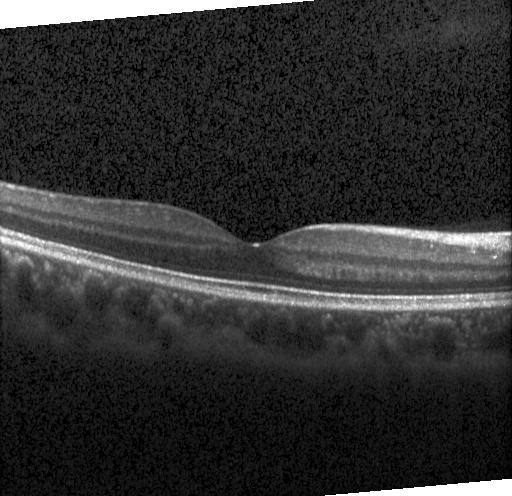
Optical coherence tomography B-scan — This B-scan demonstrates no evidence of CNV, DME, or drusen.